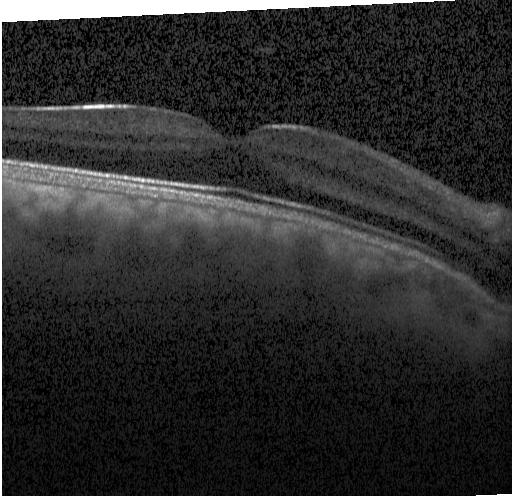 Spectral-domain OCT; retinal OCT cross-section
Finding: no choroidal neovascularization, no diabetic macular edema, and no drusen.